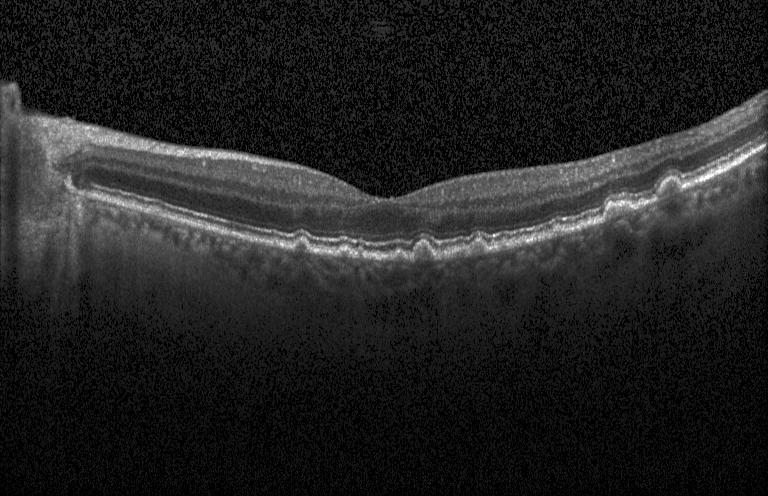
Optical coherence tomography B-scan · Heidelberg Spectralis.
Finding: sub-RPE drusenoid deposits.